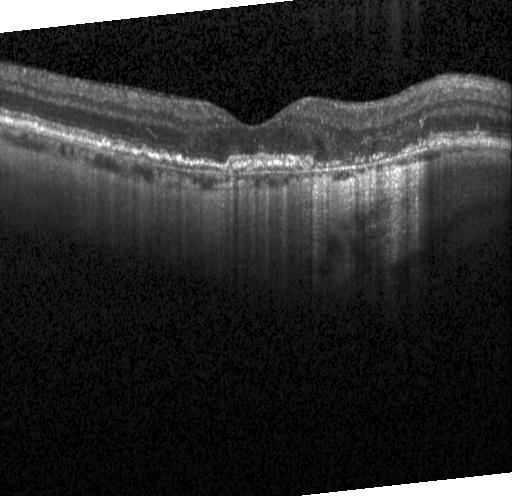

OCT B-scan showing a choroidal neovascular membrane.